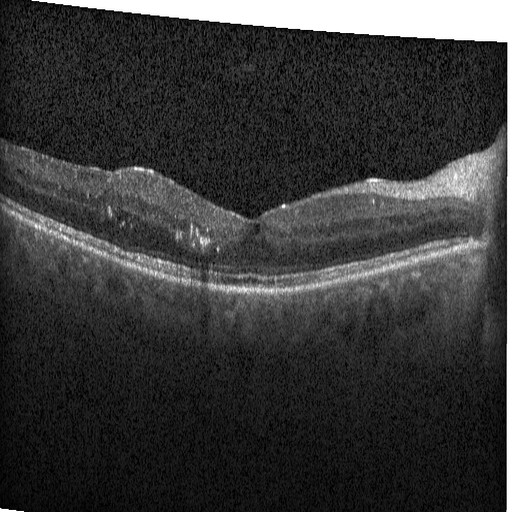 OCT finding: DME.